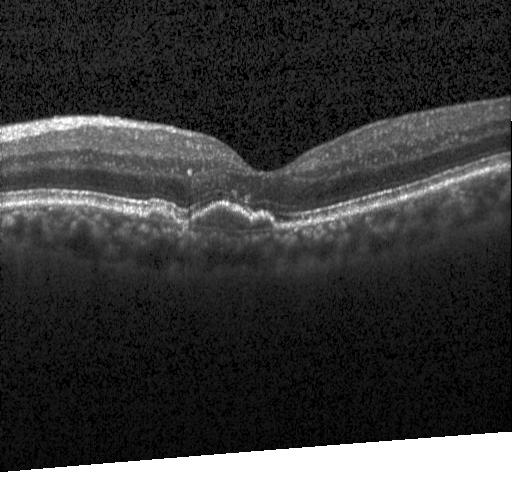 OCT line scan. Diagnosis: a choroidal neovascular membrane.